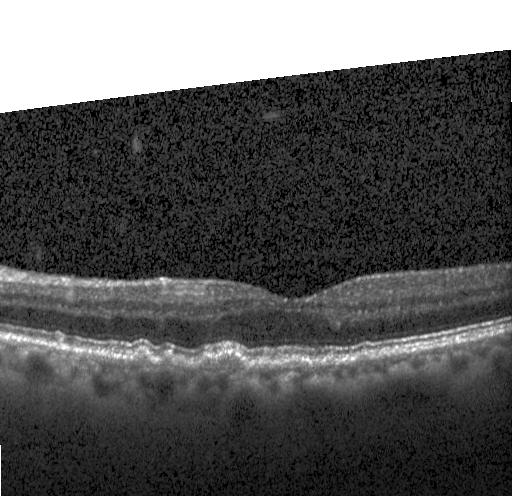 Through the macula, spectral-domain optical coherence tomography, retinal OCT B-scan. The scan shows sub-RPE drusenoid deposits.